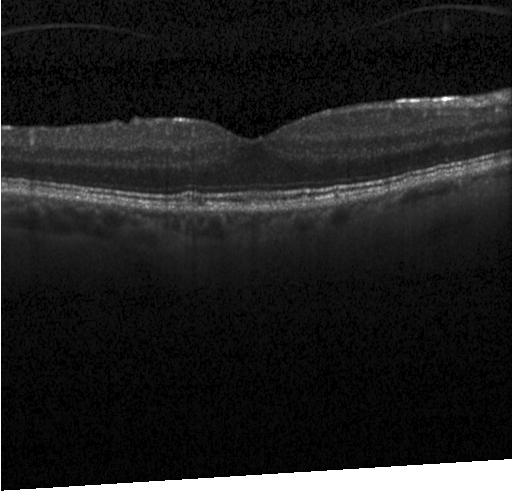

Spectral-domain OCT · horizontal scan through the fovea · instrument: Heidelberg Spectralis · OCT line scan. OCT finding: no evidence of choroidal neovascularization, diabetic macular edema, or drusen.